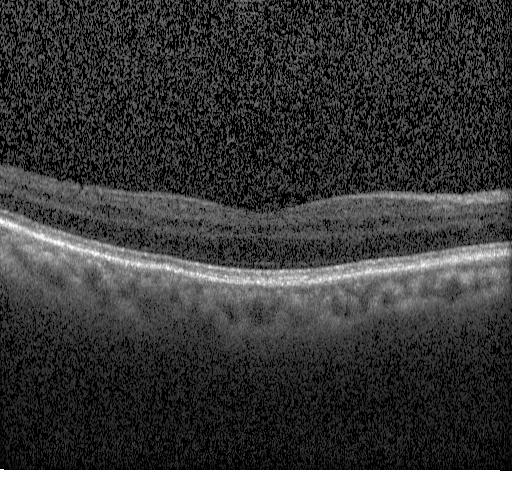
Heidelberg Spectralis OCT system, retinal OCT cross-section, spectral-domain optical coherence tomography, centered on the fovea. This B-scan demonstrates neither choroidal neovascularization, diabetic macular edema, nor drusen.